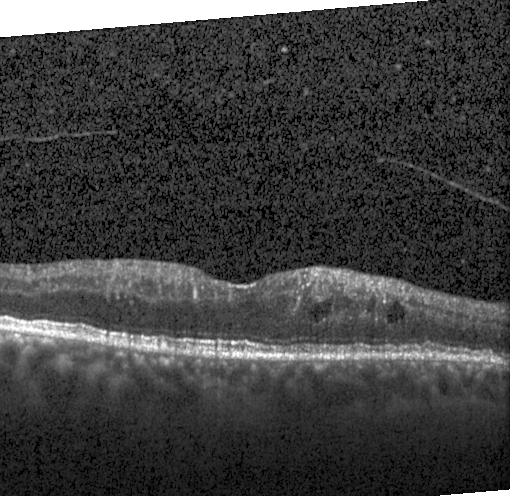
OCT finding: diabetic macular edema (DME).